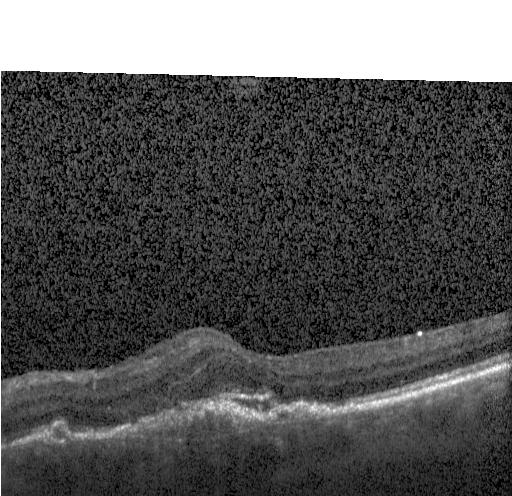

Optical coherence tomography B-scan, spectral-domain OCT. Diagnosis: a choroidal neovascular membrane.